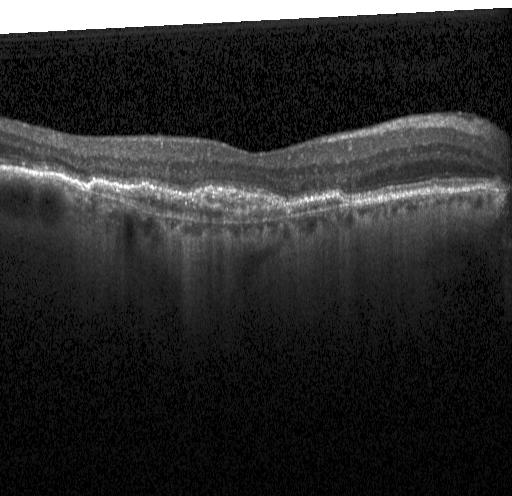 Choroidal neovascularization.